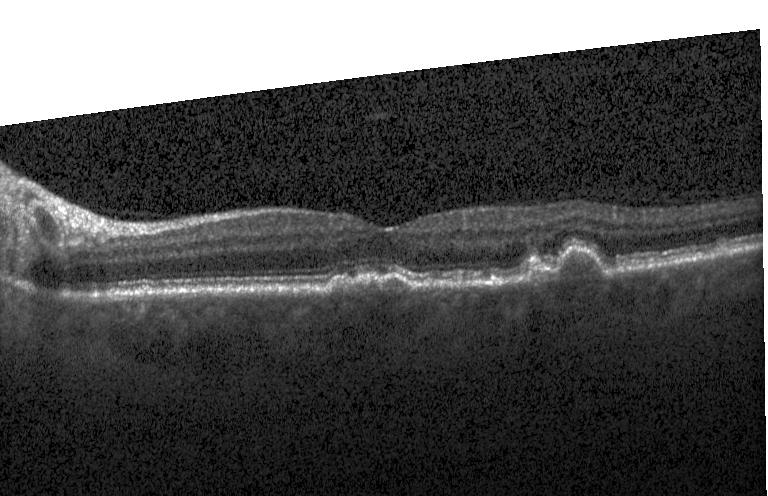

Instrument: Heidelberg Spectralis. Centered on the fovea. OCT line scan. Spectral-domain optical coherence tomography. Sub-RPE drusenoid deposits.